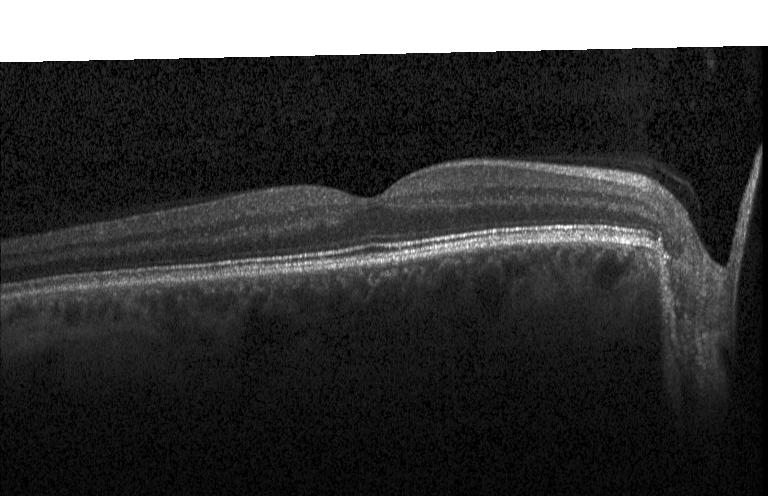 Dx: no evidence of CNV, DME, or drusen.